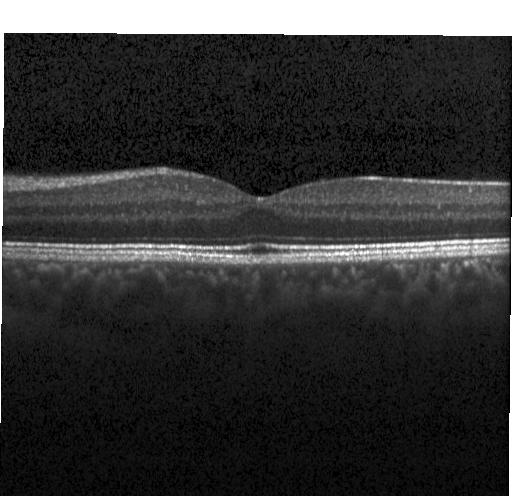 Impression: no choroidal neovascularization, no diabetic macular edema, and no drusen.